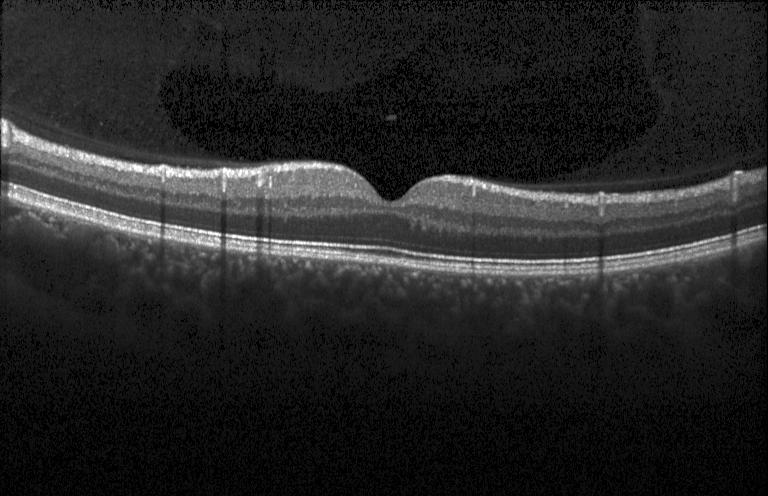
SD-OCT; OCT line scan; fovea-centered. No choroidal neovascularization, no diabetic macular edema, and no drusen.